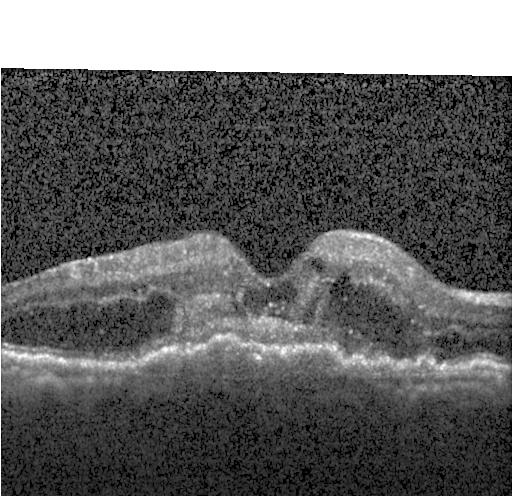
Heidelberg Spectralis; OCT B-scan; SD-OCT; centered on the fovea. Assessment: a choroidal neovascular membrane.